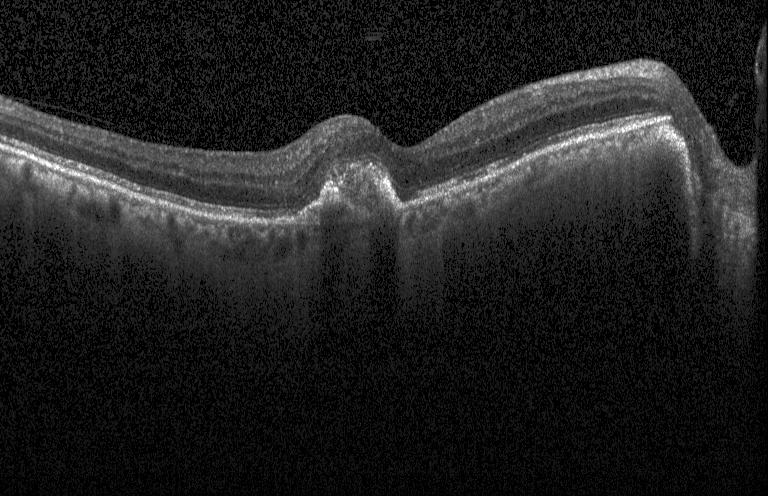 Spectral-domain optical coherence tomography. Retinal OCT B-scan — Impression: choroidal neovascularization.